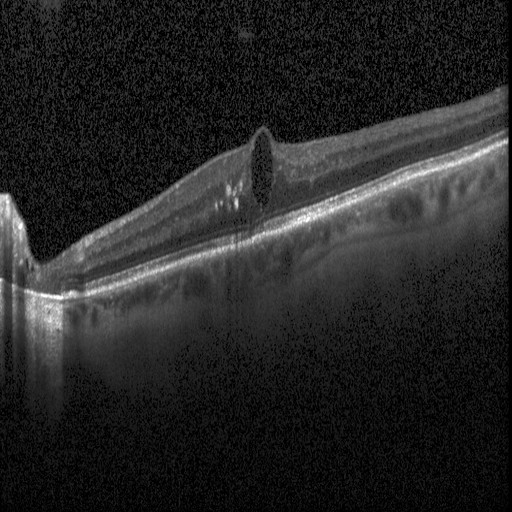

OCT B-scan · macular scan · acquired on a Heidelberg Spectralis · spectral-domain OCT
Assessment: DME.